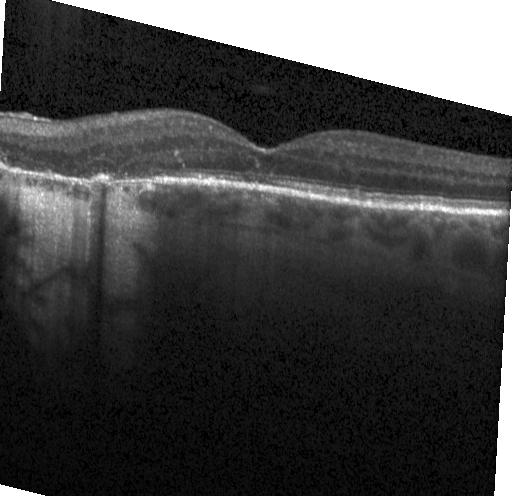 OCT line scan, spectral-domain OCT — Finding: a choroidal neovascular membrane.